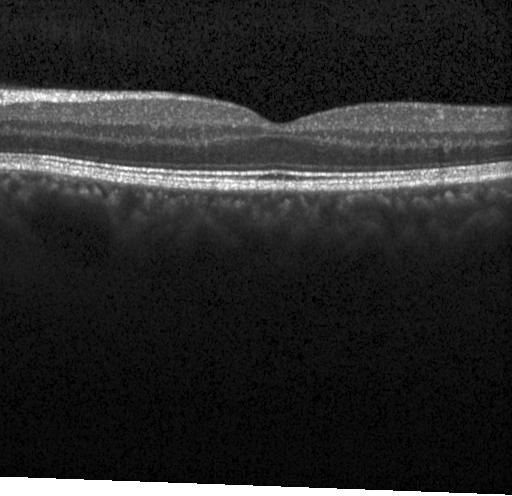 Acquired on a Heidelberg Spectralis · OCT B-scan.
Macular OCT: no evidence of choroidal neovascularization, diabetic macular edema, or drusen.